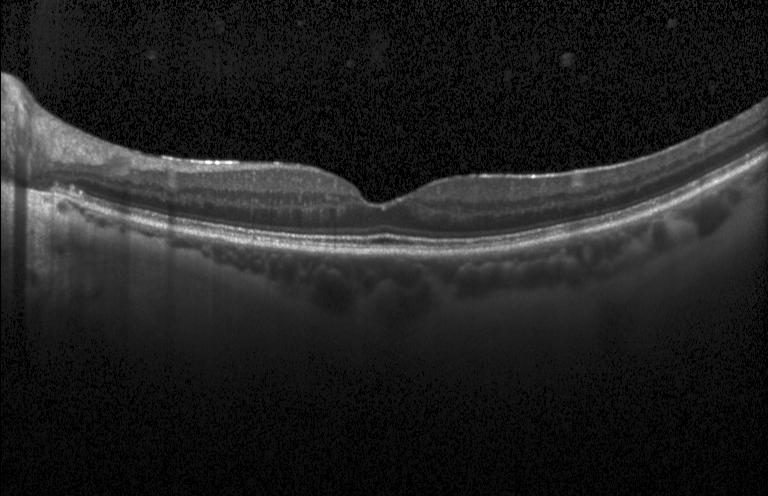
OCT B-scan; macular scan
Dx: no choroidal neovascularization, no diabetic macular edema, and no drusen.